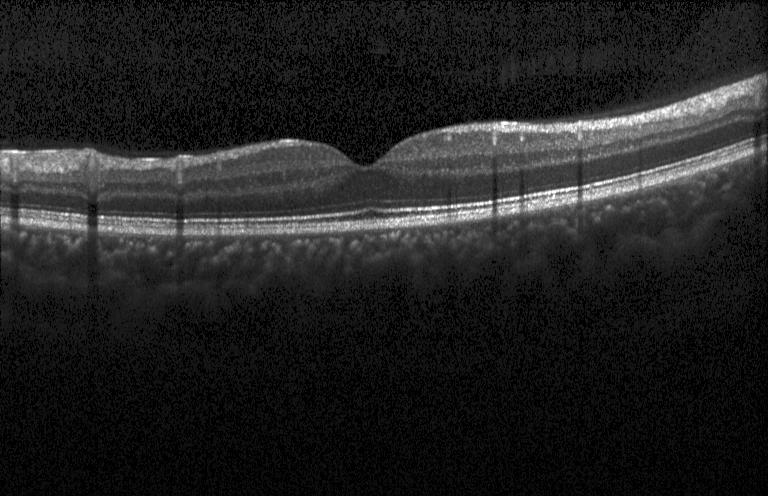

SD-OCT, Heidelberg Spectralis, OCT B-scan. Macular OCT: no evidence of CNV, DME, or drusen.